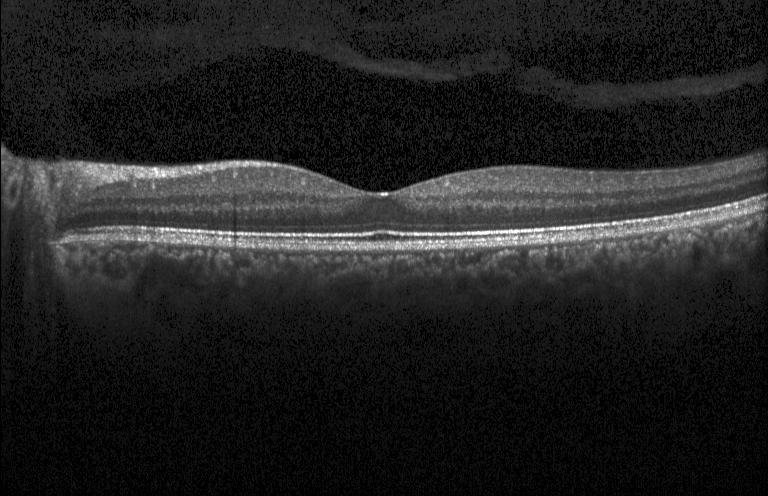
OCT B-scan. Dx: no choroidal neovascularization, no diabetic macular edema, and no drusen.